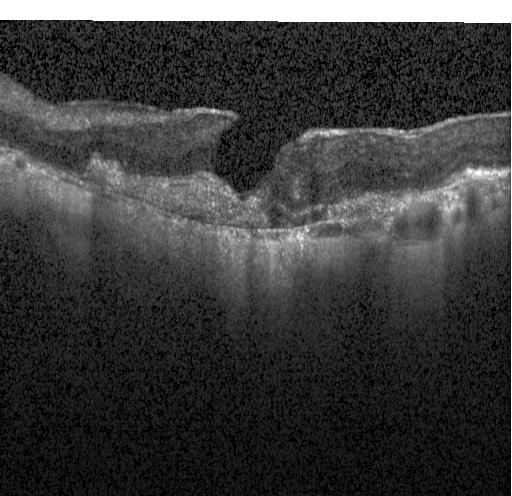

OCT scan showing choroidal neovascularization.